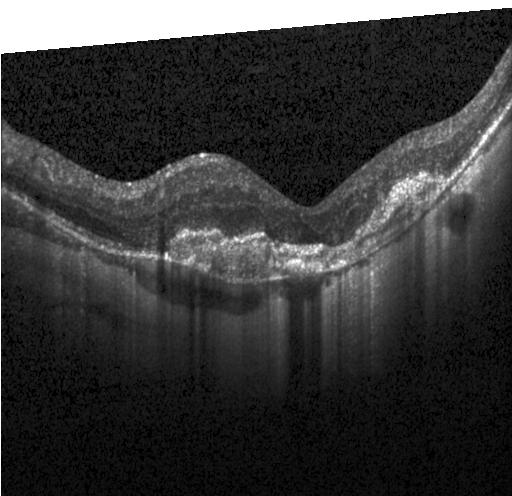
Spectral-domain optical coherence tomography, horizontal scan through the fovea, retinal OCT cross-section, acquired on a Heidelberg Spectralis.
Macular OCT: choroidal neovascularization (CNV).